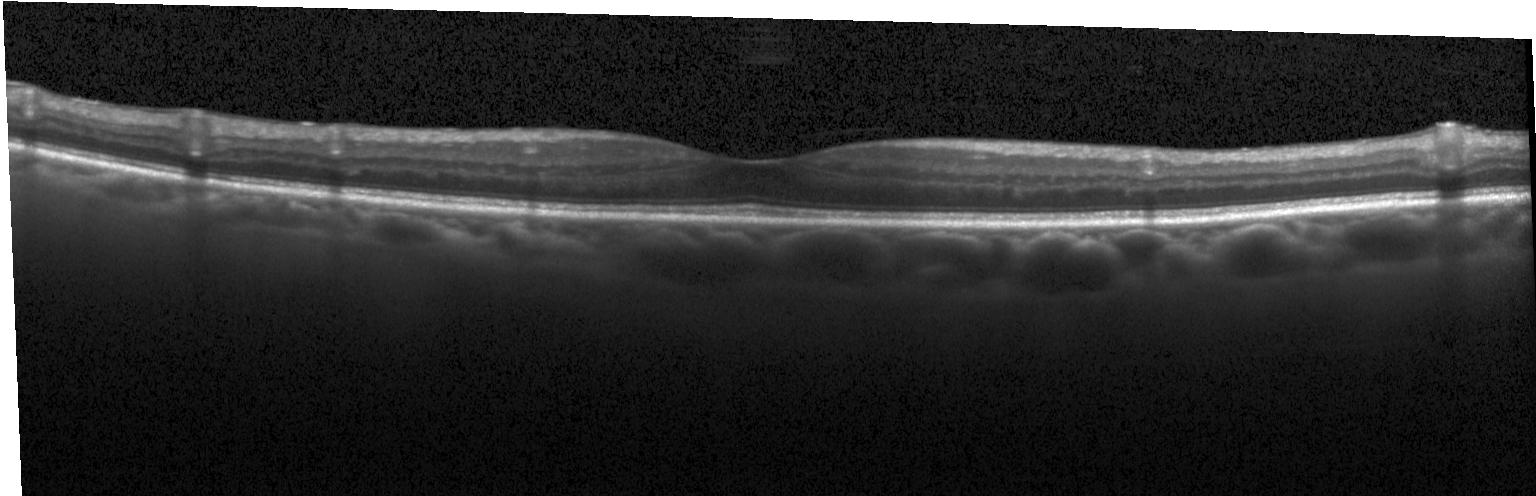 Optical coherence tomography scan · through the macula
Diagnosis: neither choroidal neovascularization, diabetic macular edema, nor drusen.